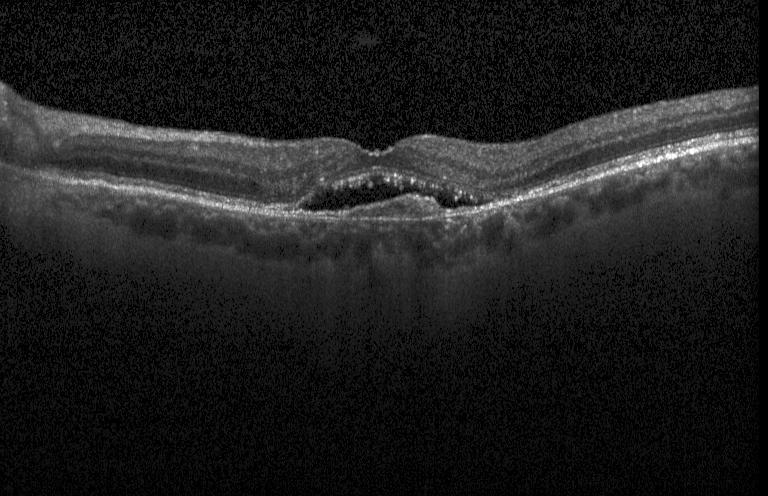 Optical coherence tomography scan.
Finding: a choroidal neovascular membrane.